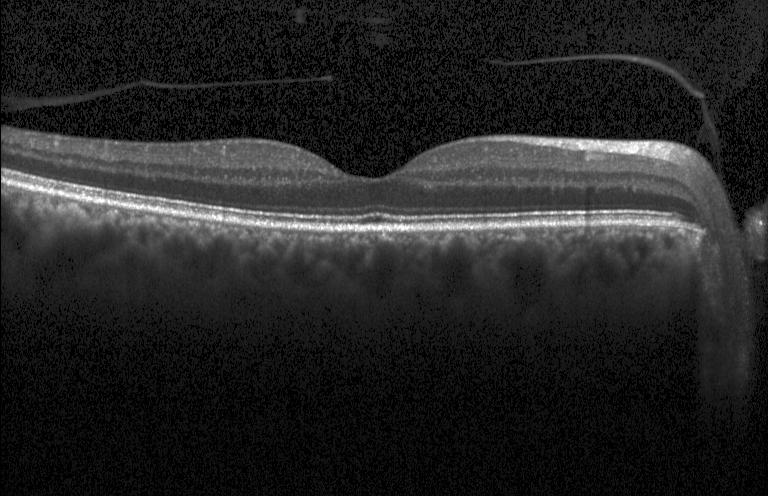
Centered on the fovea. Retinal OCT cross-section. Spectral-domain OCT.
Dx: no CNV, no DME, and no drusen.